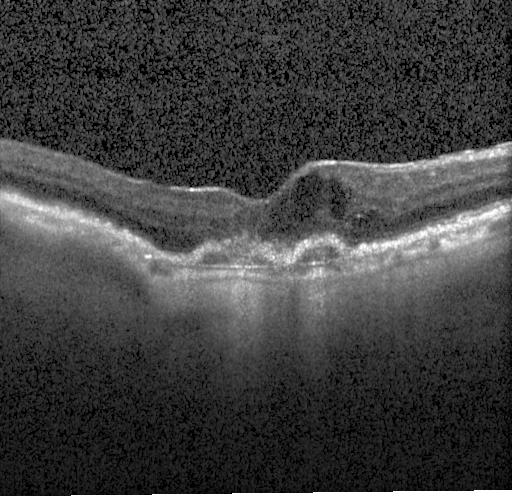 Finding: choroidal neovascularization (CNV).